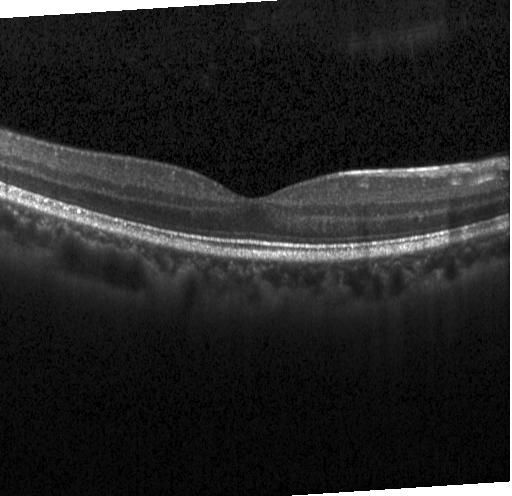

Spectral-domain optical coherence tomography, fovea-centered, retinal OCT B-scan.
Diagnosis: no choroidal neovascularization, diabetic macular edema, or drusen.